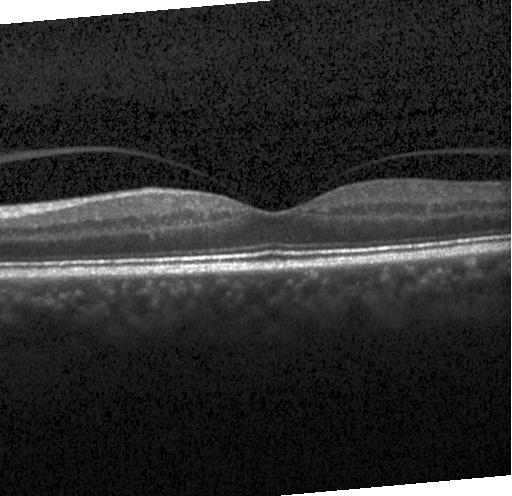
Optical coherence tomography scan; through the macula.
Assessment: neither CNV, DME, nor drusen.